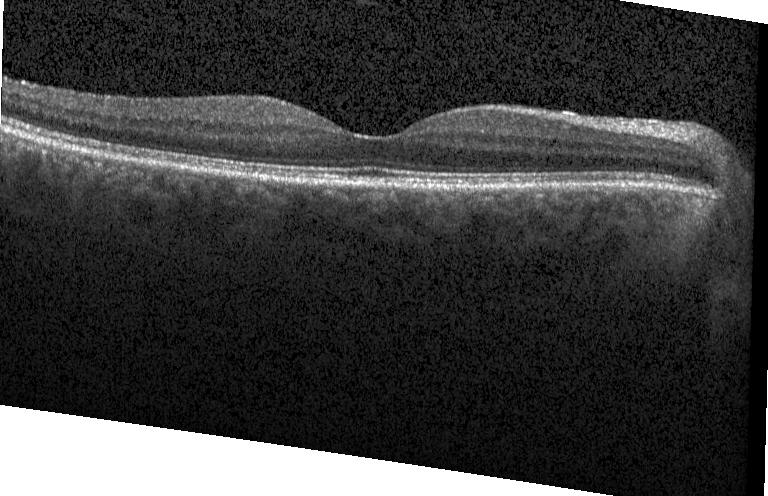

Optical coherence tomography B-scan — Assessment: no choroidal neovascularization, diabetic macular edema, or drusen.